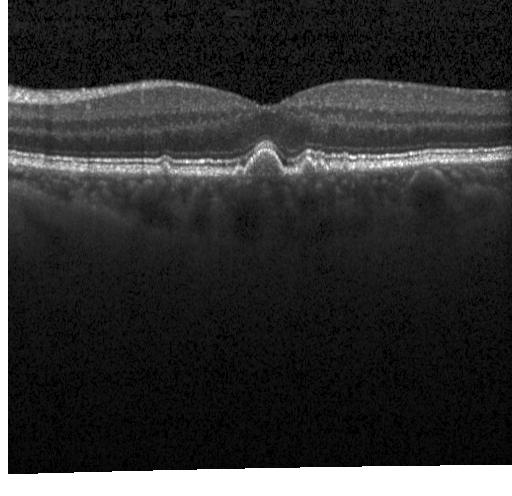
The scan shows multiple drusen.